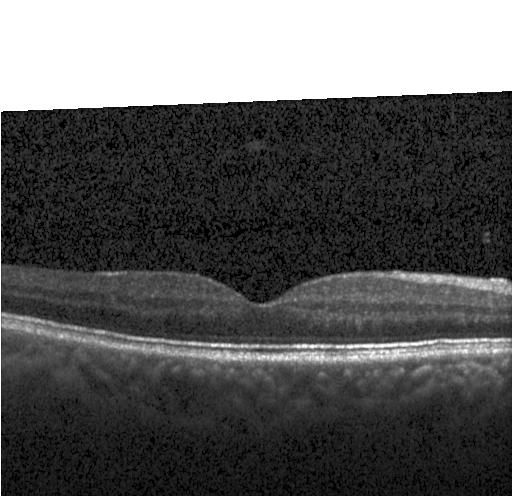 Optical coherence tomography B-scan.
Diagnosis: no choroidal neovascularization, diabetic macular edema, or drusen.